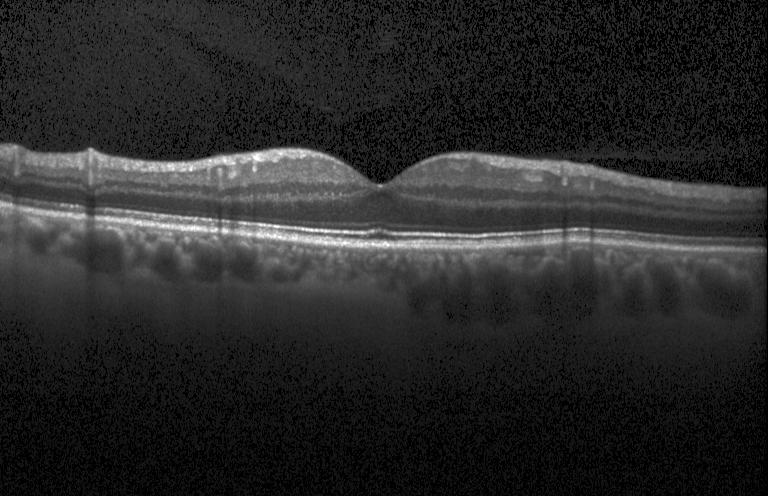 Heidelberg Spectralis OCT system · optical coherence tomography B-scan · spectral-domain OCT · horizontal scan through the fovea
Impression: no evidence of choroidal neovascularization, diabetic macular edema, or drusen.